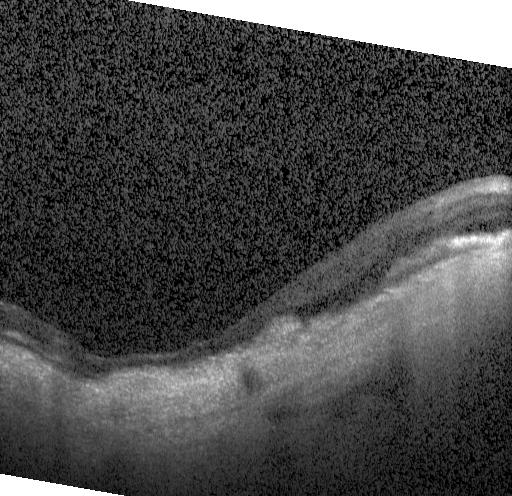

SD-OCT; acquired on a Heidelberg Spectralis; OCT B-scan; through the macula.
Diagnosis: CNV.